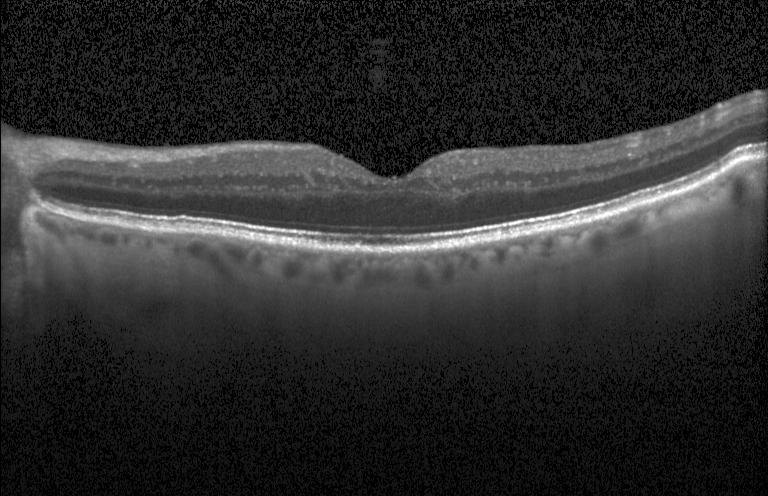
Spectral-domain OCT B-scan: no choroidal neovascularization, no diabetic macular edema, and no drusen.